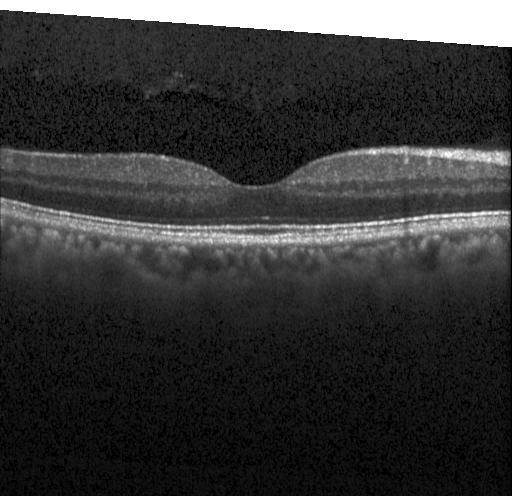

OCT B-scan
Macular OCT: no CNV, no DME, and no drusen.